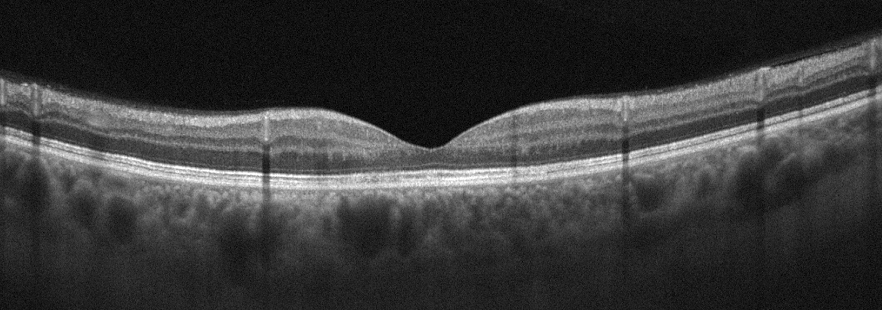

Macular OCT demonstrating no AMD, DME, ERM, RAO, RVO, or VID.